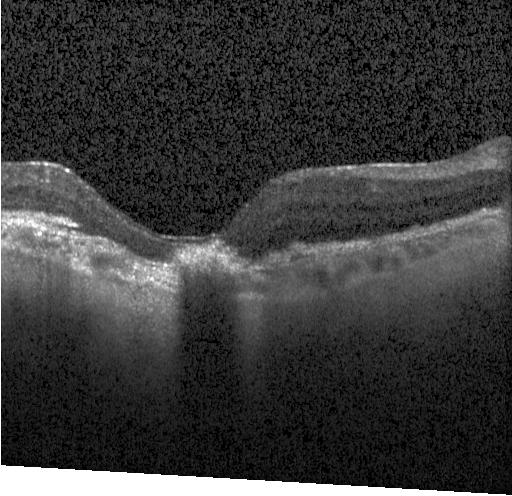 Retinal OCT cross-section — Dx: CNV.